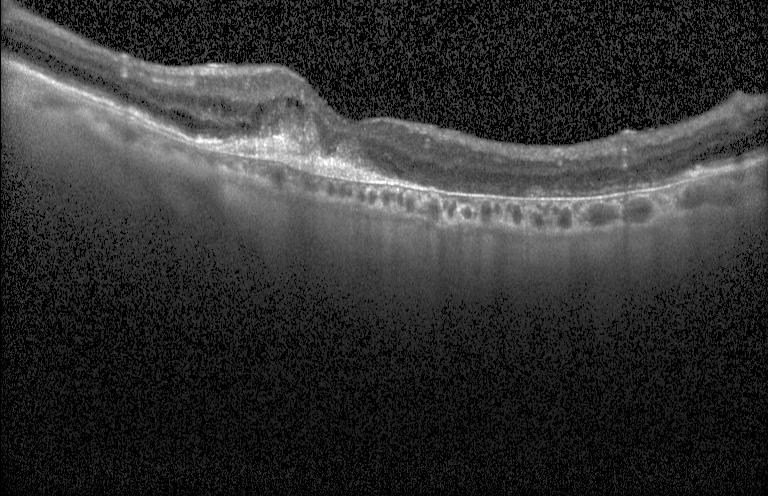

Macular OCT demonstrating a choroidal neovascular membrane.